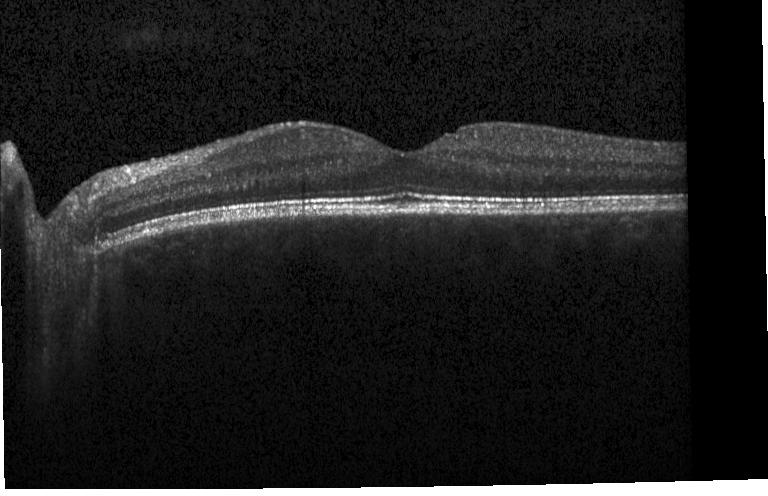

SD-OCT. Optical coherence tomography scan. Diagnosis: no evidence of CNV, DME, or drusen.